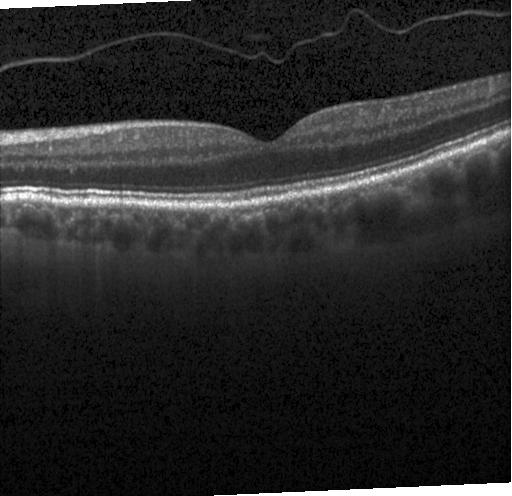 Optical coherence tomography scan — Assessment: no evidence of CNV, DME, or drusen.